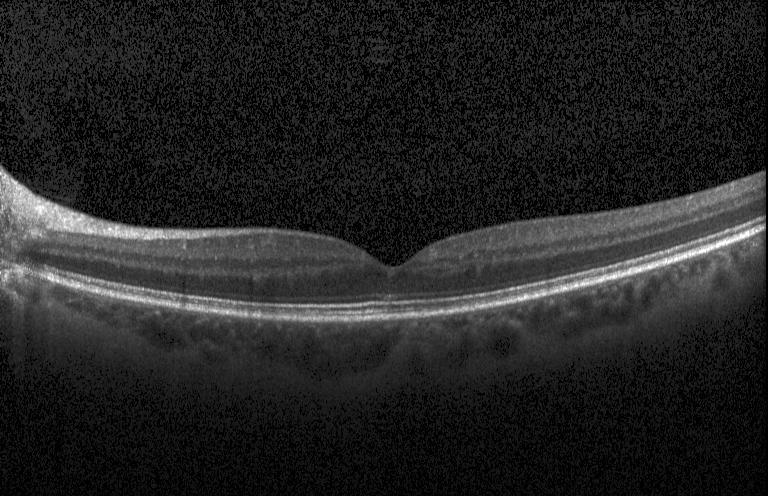 Through the macula · OCT B-scan · SD-OCT. Impression: no choroidal neovascularization, diabetic macular edema, or drusen.